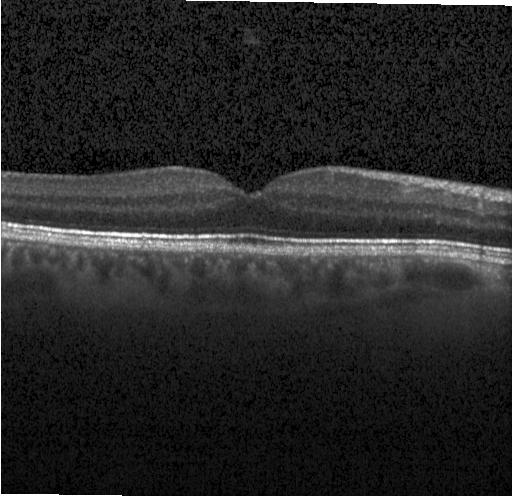 This B-scan demonstrates no choroidal neovascularization, diabetic macular edema, or drusen.